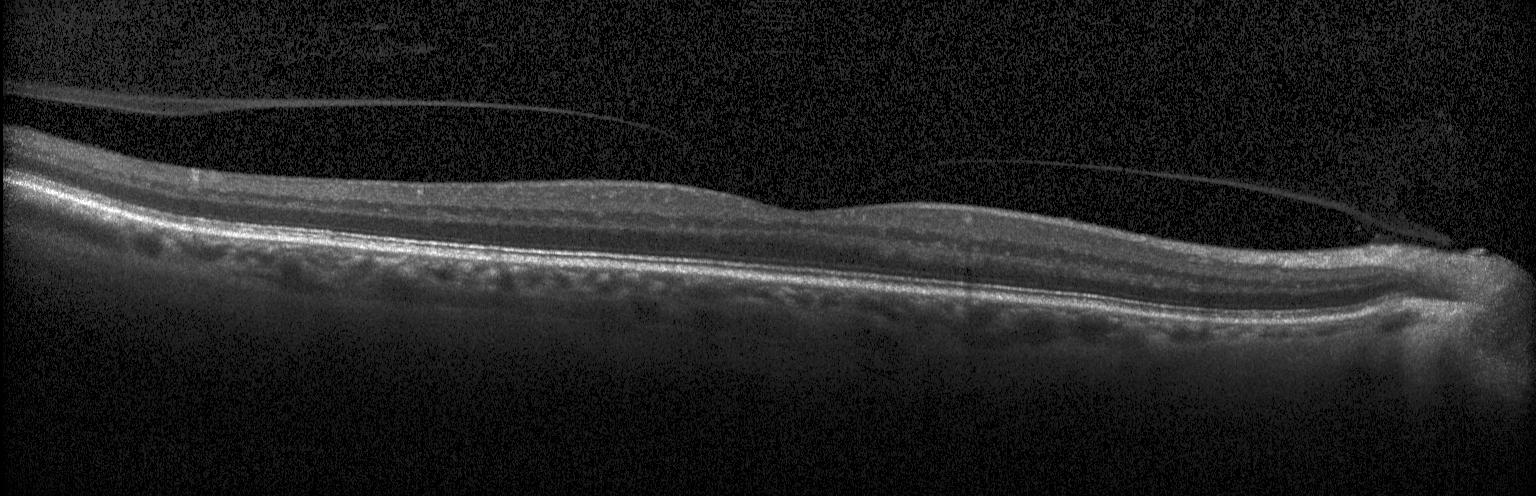
Impression: no CNV, no DME, and no drusen.